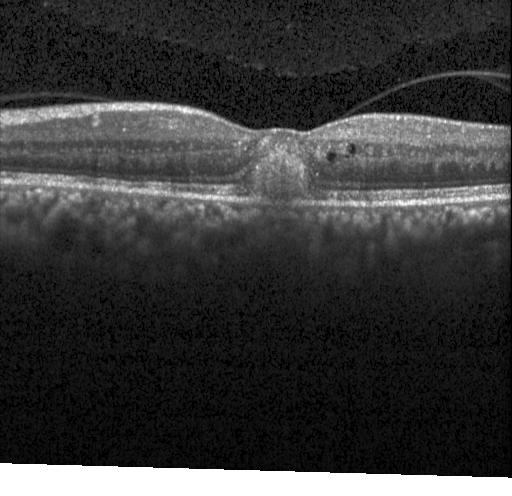
Impression: a choroidal neovascular membrane.